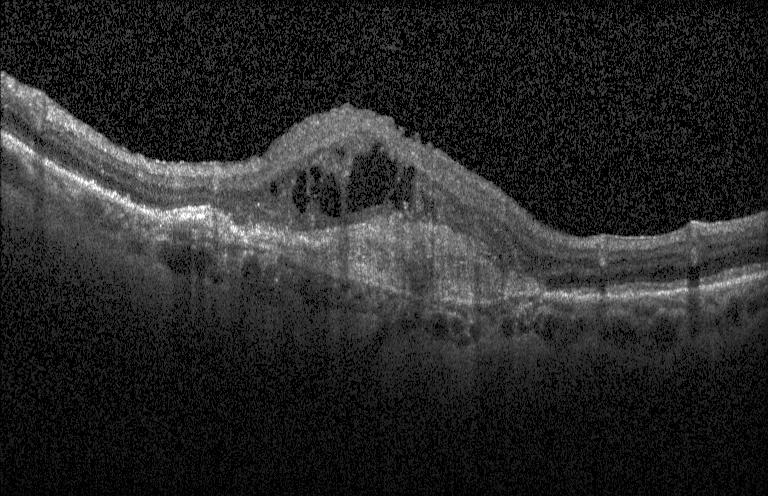
Spectral-domain OCT · OCT B-scan
Diagnosis: choroidal neovascularization.